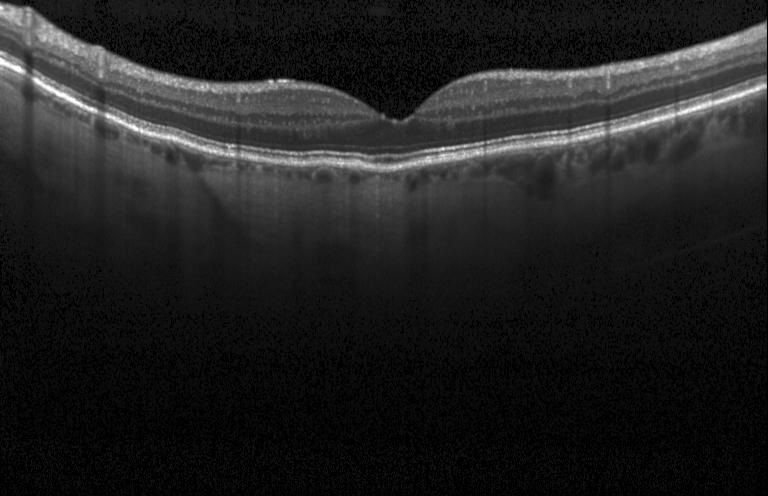 Diagnosis: no evidence of choroidal neovascularization, diabetic macular edema, or drusen.